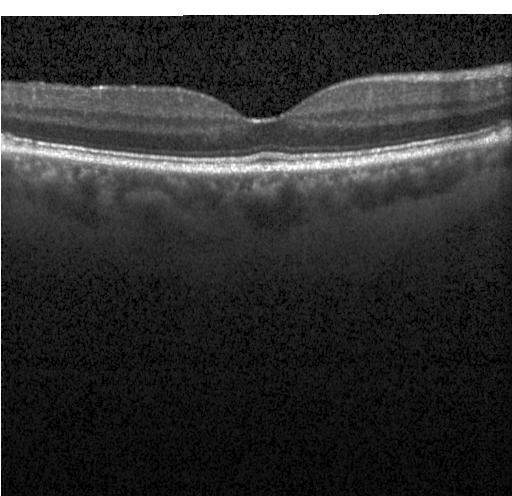
Retinal OCT cross-section. Acquired on a Heidelberg Spectralis. No choroidal neovascularization, no diabetic macular edema, and no drusen.